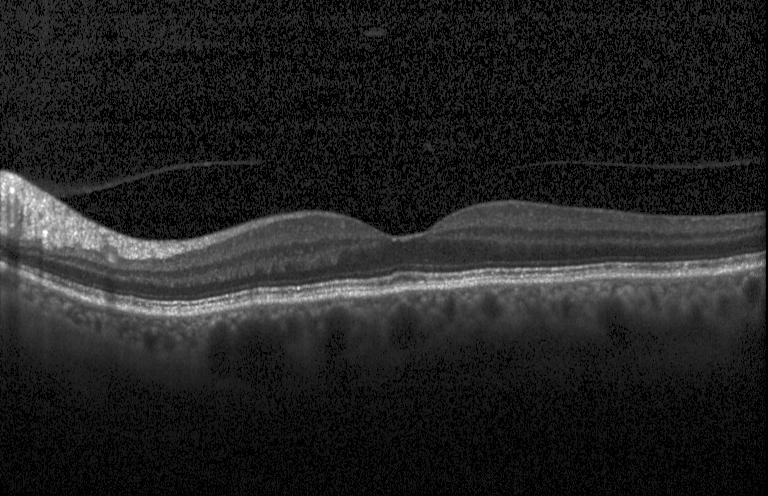
OCT B-scan showing no choroidal neovascularization, no diabetic macular edema, and no drusen.